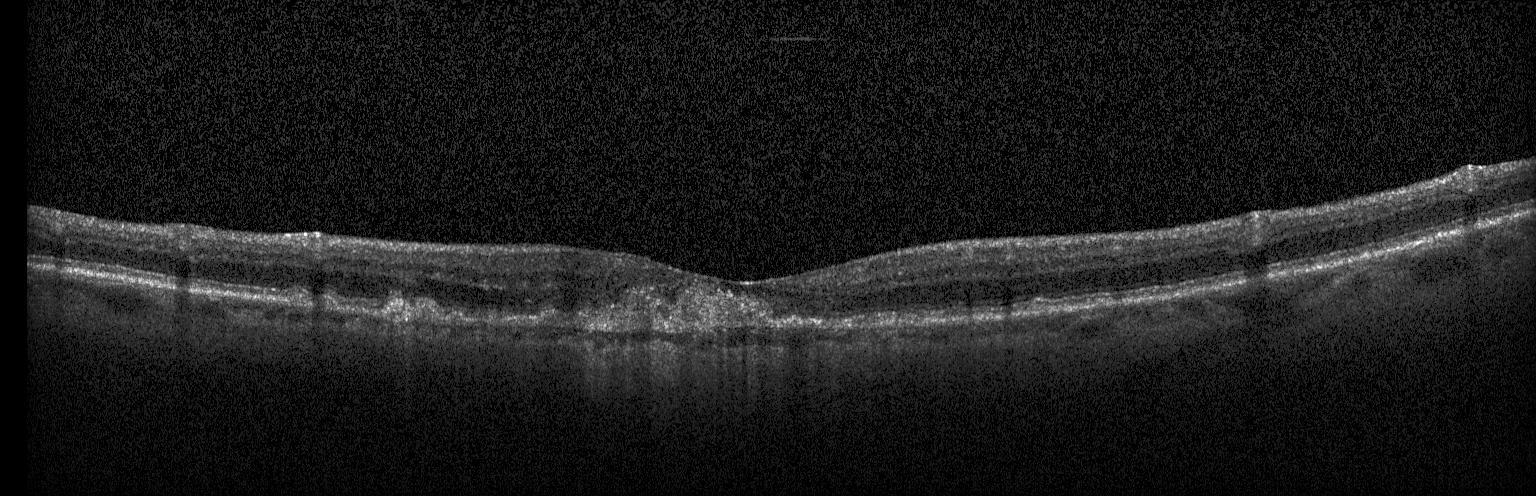 OCT line scan, macular scan, Heidelberg Spectralis. Finding: choroidal neovascularization.